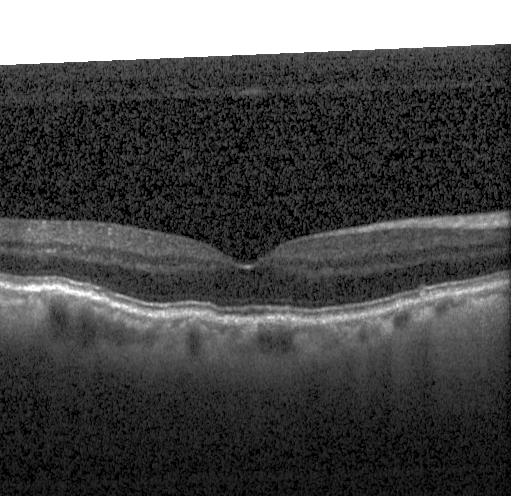

Heidelberg Spectralis OCT system; macular scan; optical coherence tomography scan; spectral-domain optical coherence tomography. The scan shows multiple drusen.